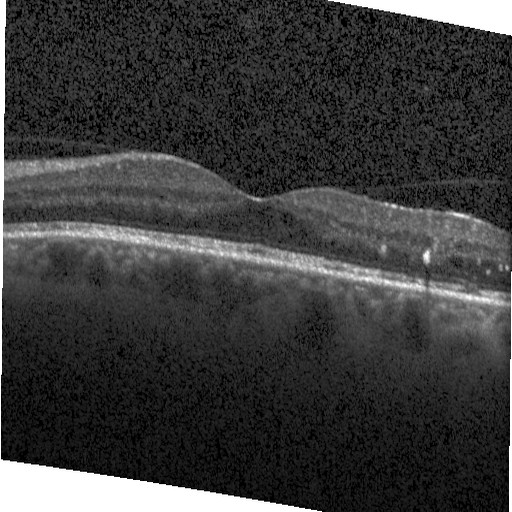

Retinal OCT cross-section
Finding: diabetic macular edema (DME).